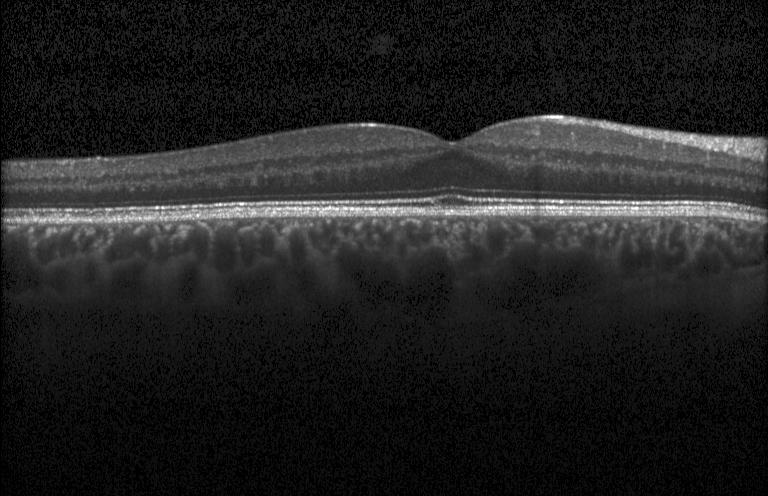
Horizontal scan through the fovea · spectral-domain OCT · optical coherence tomography scan.
No choroidal neovascularization, no diabetic macular edema, and no drusen.